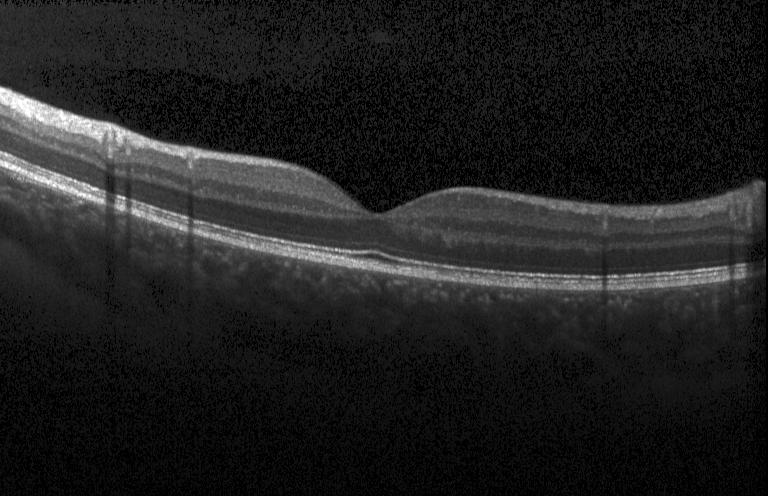

Heidelberg Spectralis; horizontal scan through the fovea; OCT line scan; spectral-domain OCT — The scan shows no choroidal neovascularization, no diabetic macular edema, and no drusen.